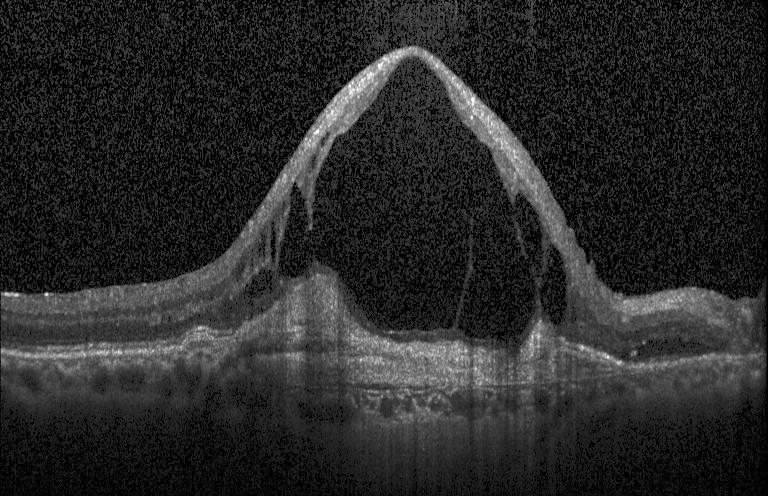

Fovea-centered. OCT B-scan. Heidelberg Spectralis.
Macular OCT: choroidal neovascularization.